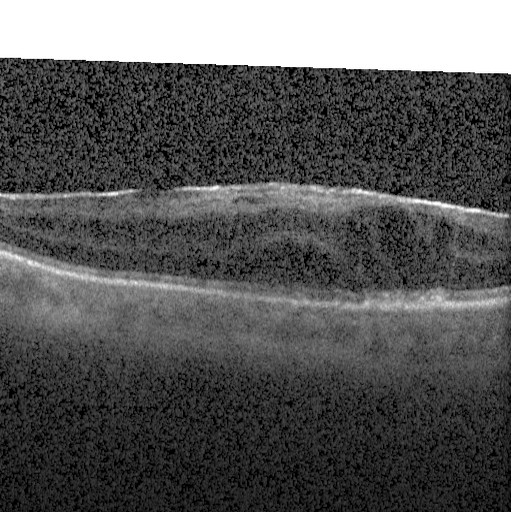

Macular OCT: DME.